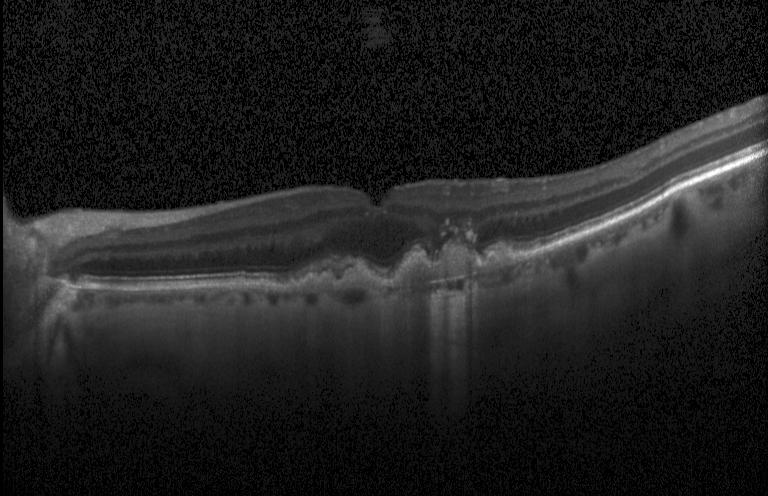

OCT scan showing multiple drusen.